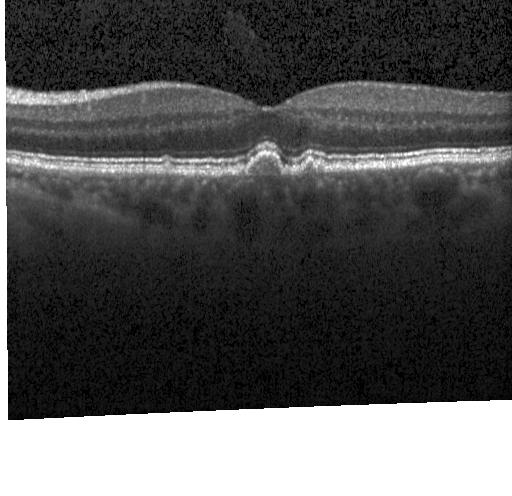
Optical coherence tomography scan
This B-scan demonstrates sub-RPE drusenoid deposits.